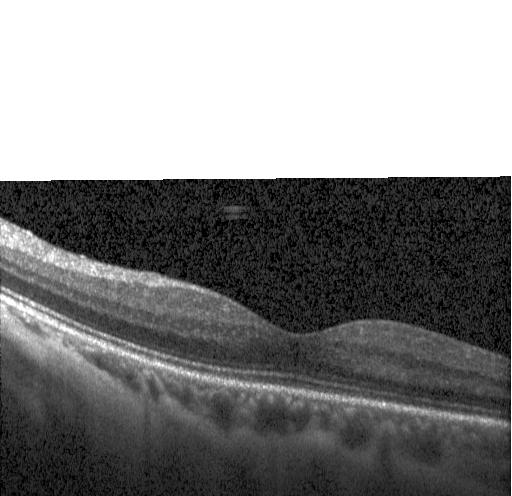
Retinal OCT cross-section showing no choroidal neovascularization, no diabetic macular edema, and no drusen.